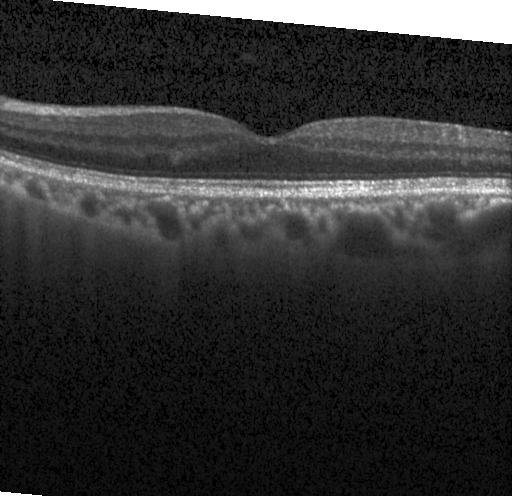

This B-scan demonstrates neither choroidal neovascularization, diabetic macular edema, nor drusen.